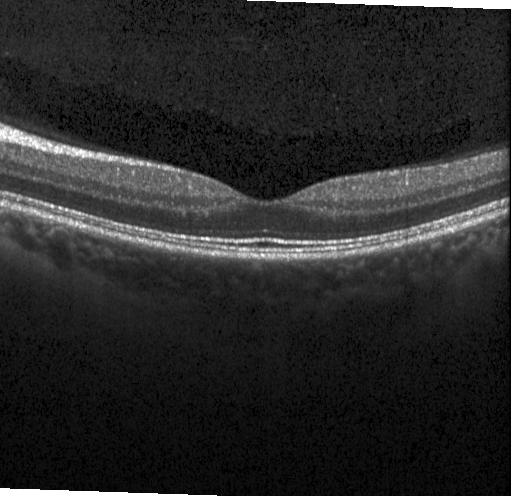
Centered on the fovea, OCT B-scan — OCT finding: no evidence of CNV, DME, or drusen.